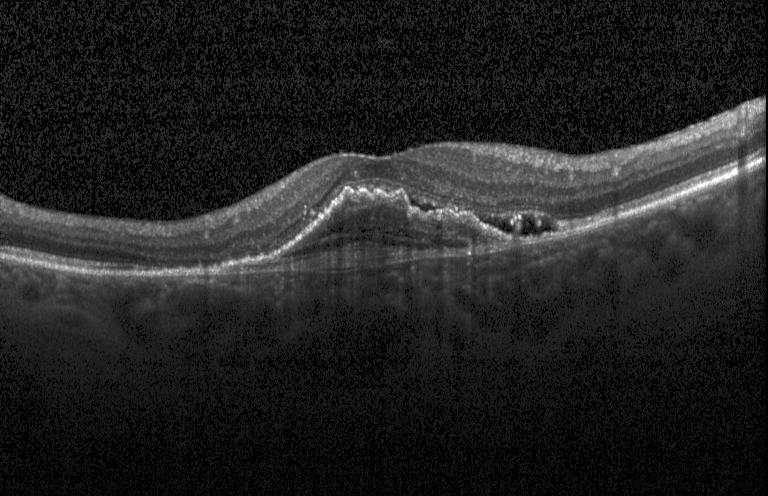 OCT B-scan — This B-scan demonstrates CNV.